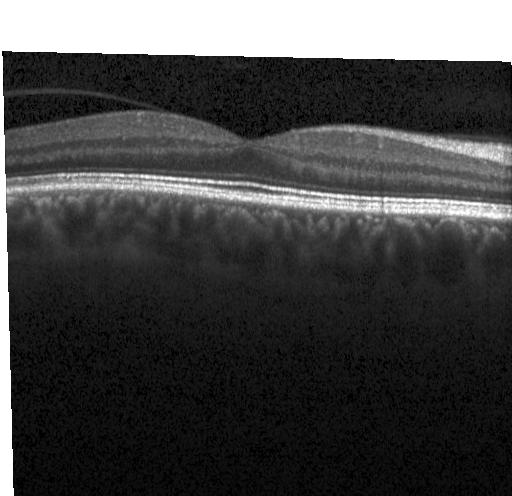 Spectral-domain OCT B-scan: no evidence of choroidal neovascularization, diabetic macular edema, or drusen.